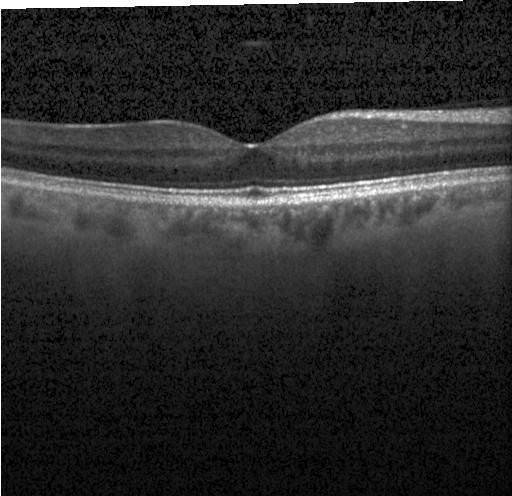 OCT B-scan showing neither choroidal neovascularization, diabetic macular edema, nor drusen.